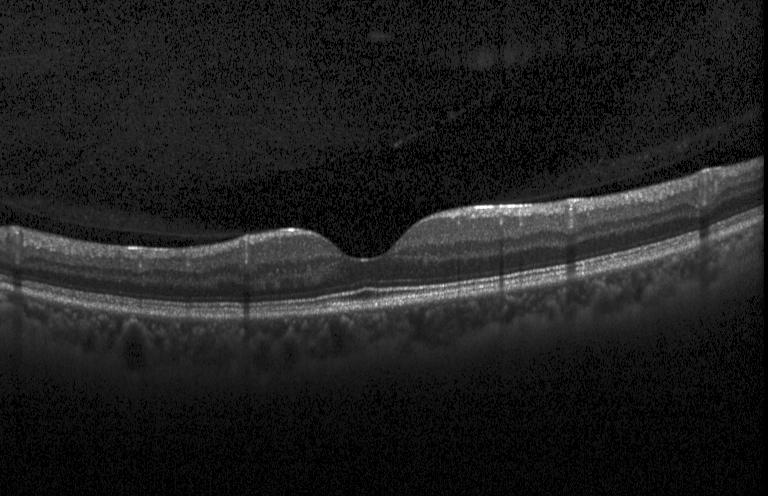

Macular OCT demonstrating no evidence of CNV, DME, or drusen.